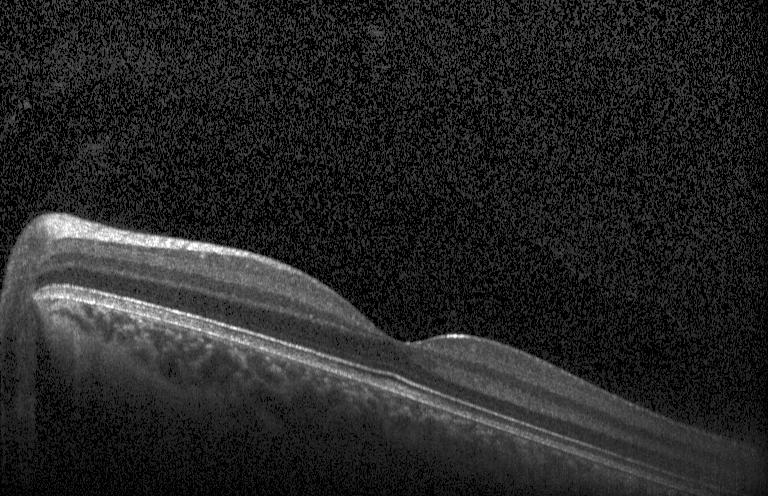
Optical coherence tomography scan.
Neither choroidal neovascularization, diabetic macular edema, nor drusen.